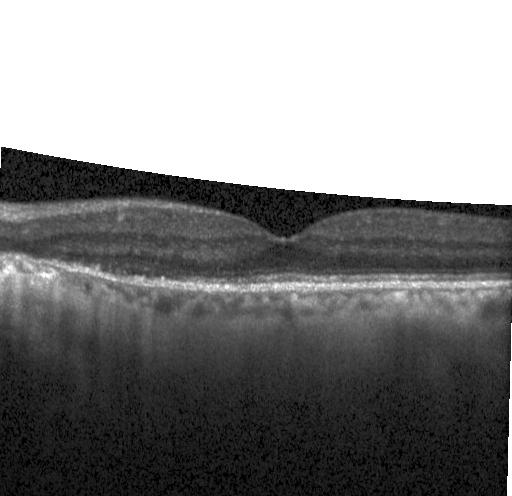

OCT line scan — Neither choroidal neovascularization, diabetic macular edema, nor drusen.